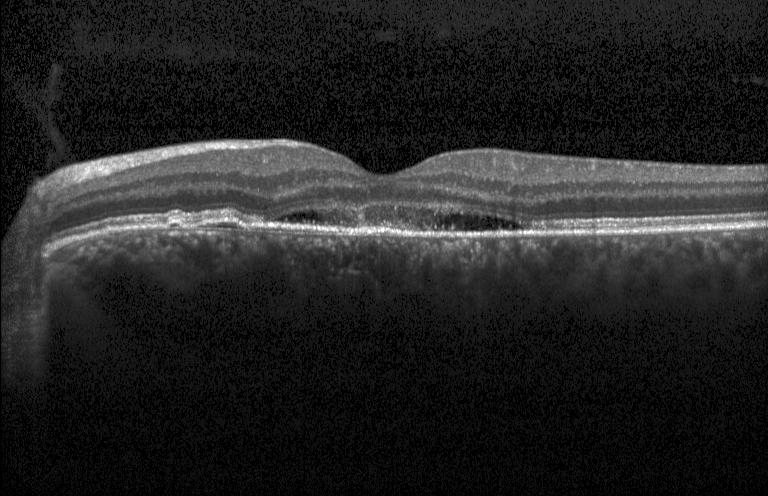
Heidelberg Spectralis · through the macula · optical coherence tomography scan. Dx: a choroidal neovascular membrane.